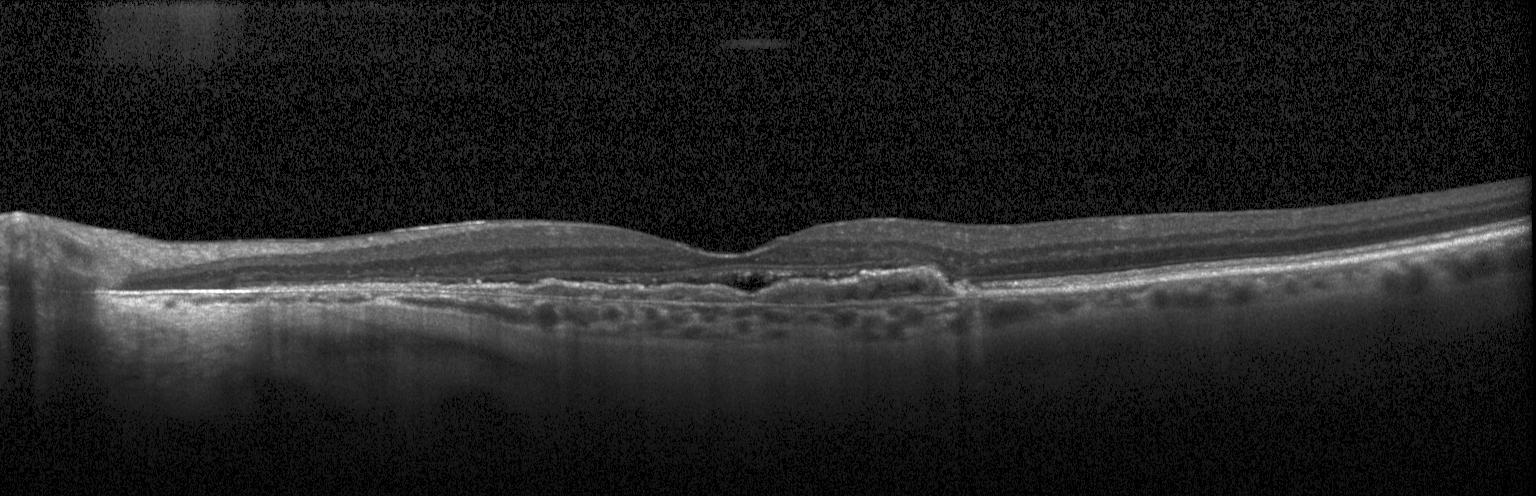 Retinal OCT B-scan; spectral-domain OCT; Heidelberg Spectralis — Finding: CNV.